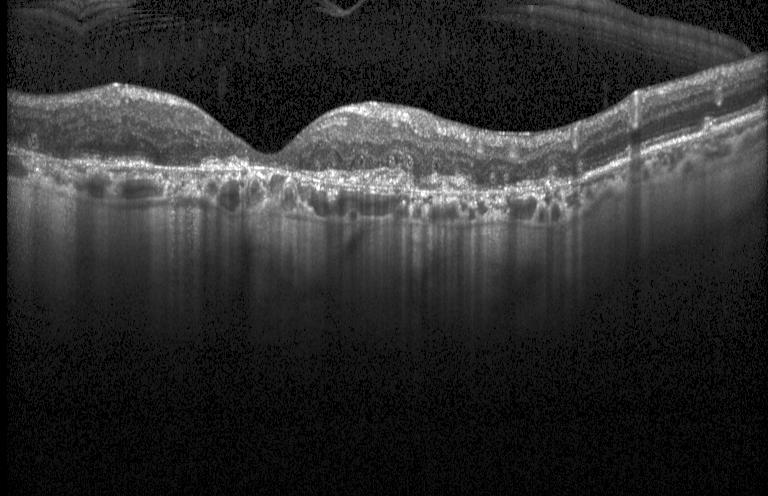 Spectral-domain OCT. OCT B-scan.
A choroidal neovascular membrane.